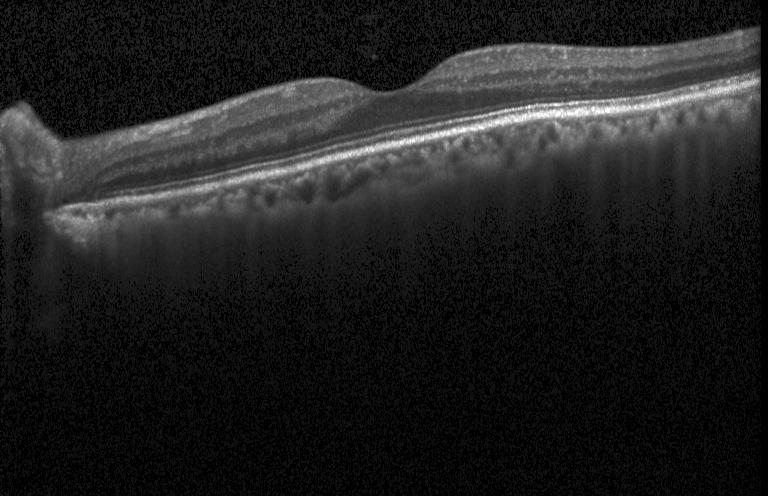
Instrument: Heidelberg Spectralis, macular scan, retinal OCT B-scan
Assessment: no evidence of choroidal neovascularization, diabetic macular edema, or drusen.